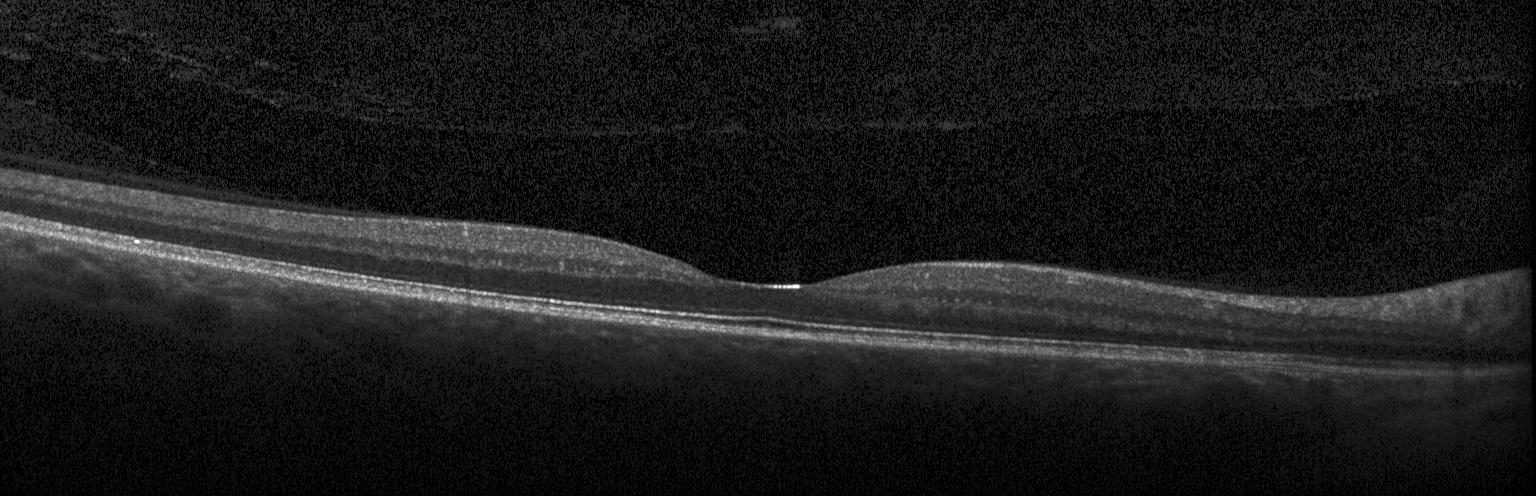
Impression: neither choroidal neovascularization, diabetic macular edema, nor drusen.